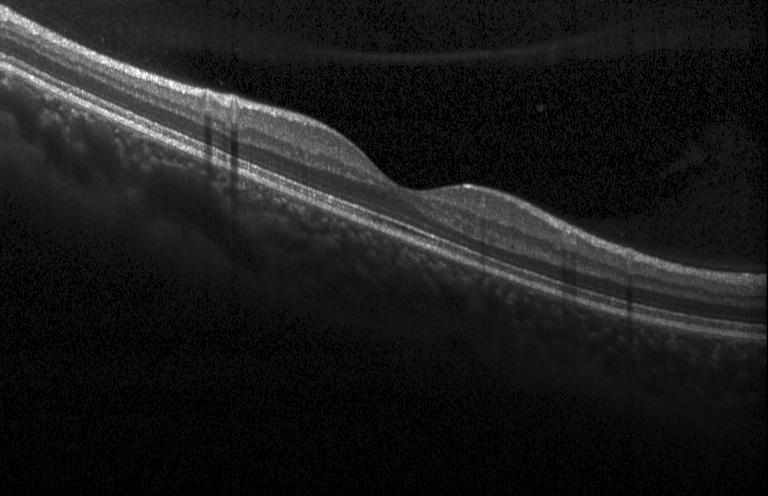 Spectral-domain OCT · optical coherence tomography B-scan.
Finding: neither choroidal neovascularization, diabetic macular edema, nor drusen.